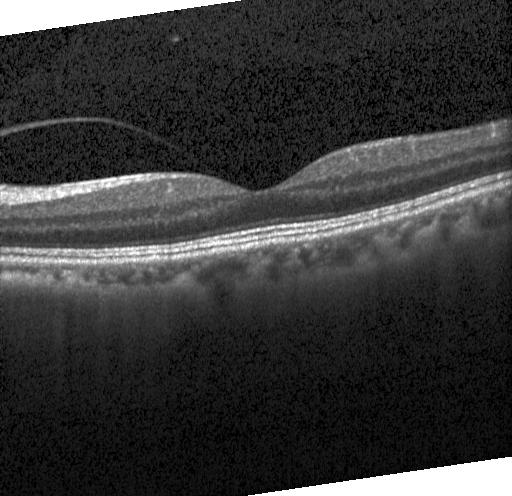

Retinal OCT B-scan; Heidelberg Spectralis OCT system; spectral-domain OCT; horizontal scan through the fovea — Assessment: no evidence of choroidal neovascularization, diabetic macular edema, or drusen.